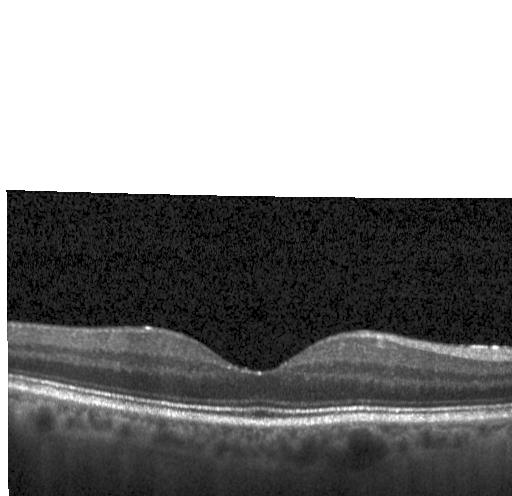

OCT B-scan.
Diagnosis: no evidence of choroidal neovascularization, diabetic macular edema, or drusen.